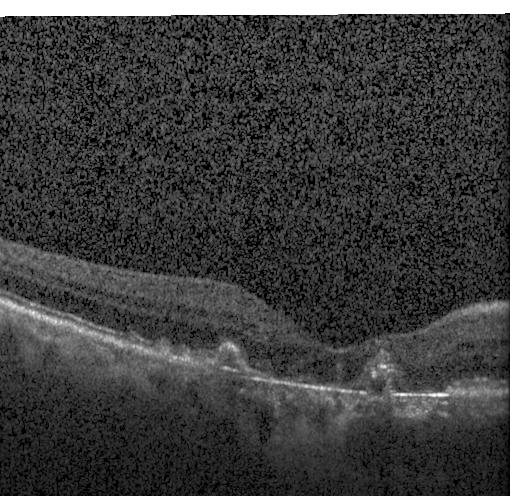

Retinal OCT cross-section; macular scan; SD-OCT
Assessment: a choroidal neovascular membrane.